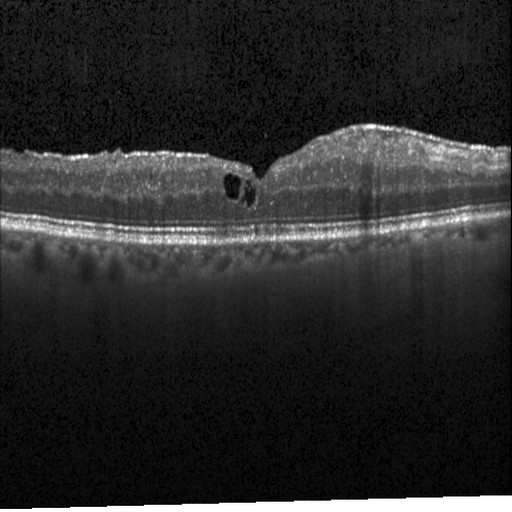
Retinal OCT cross-section.
Diagnosis: DME.